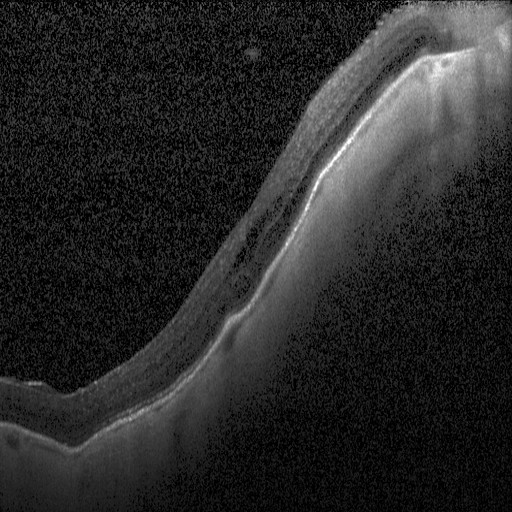 Optical coherence tomography scan. Spectral-domain optical coherence tomography. Acquired on a Heidelberg Spectralis. Horizontal scan through the fovea
Diagnosis: diabetic macular edema (DME).